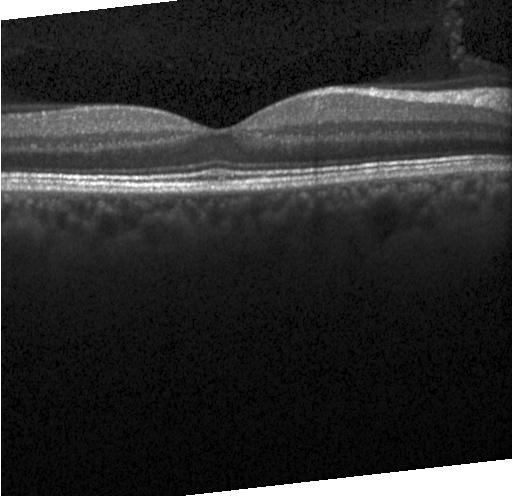
Retinal OCT cross-section showing no evidence of choroidal neovascularization, diabetic macular edema, or drusen.